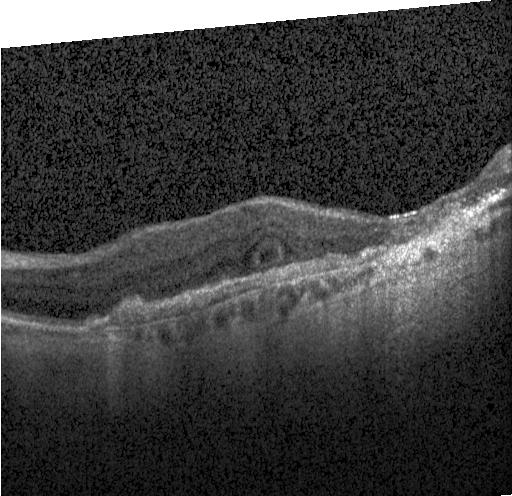 OCT scan showing a choroidal neovascular membrane.